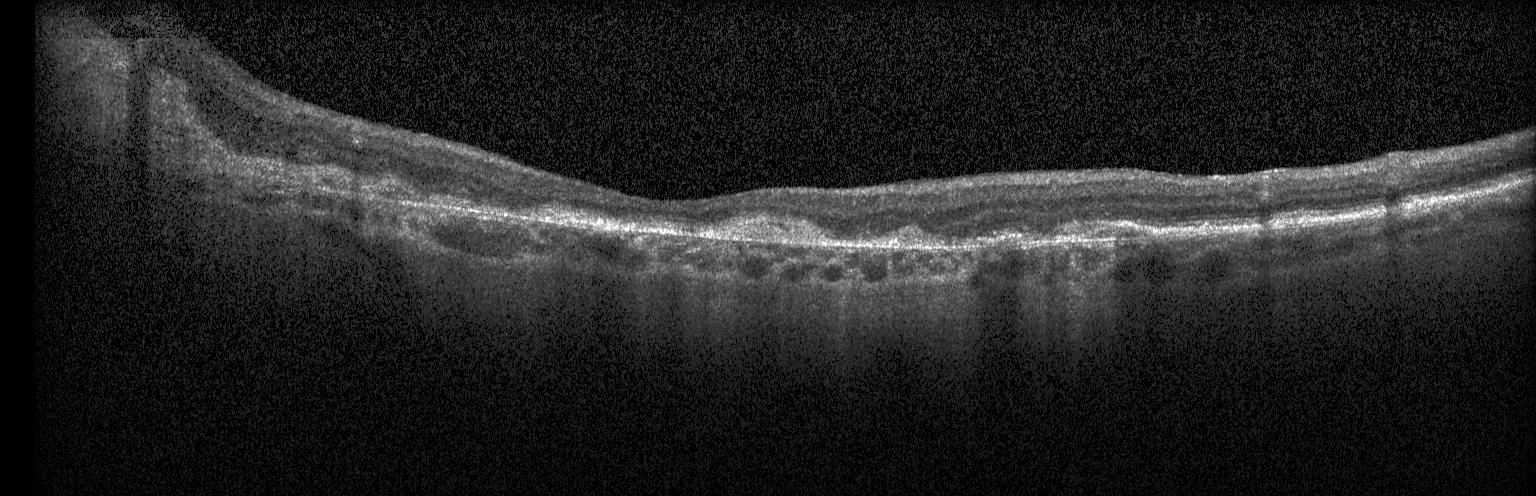
Horizontal scan through the fovea, Heidelberg Spectralis, retinal OCT cross-section, spectral-domain OCT. Assessment: a choroidal neovascular membrane.